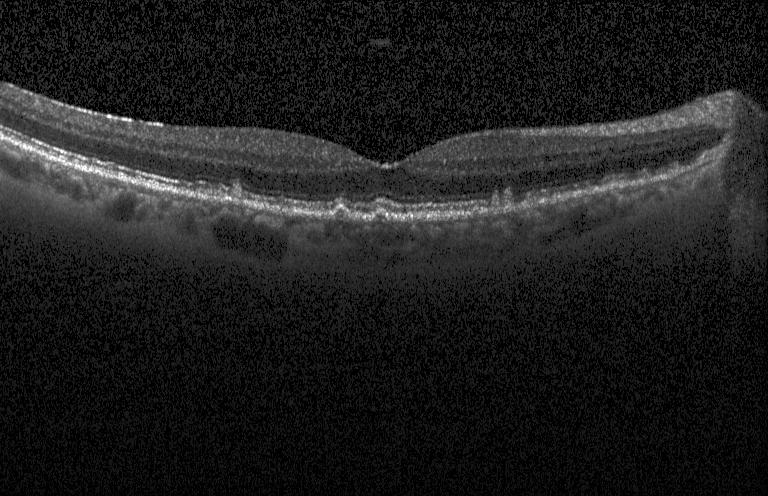 Heidelberg Spectralis · SD-OCT · optical coherence tomography scan.
The scan shows multiple drusen.